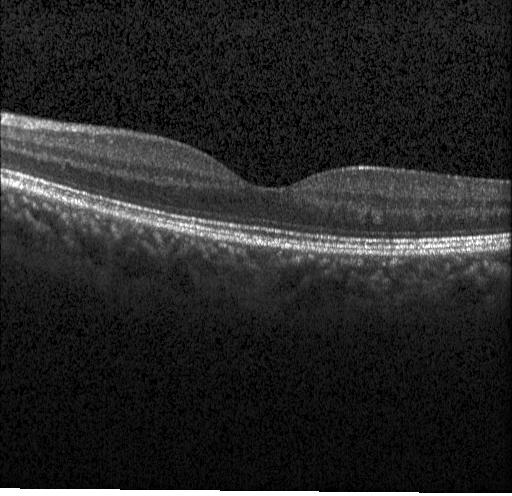 Spectral-domain OCT. Acquired on a Heidelberg Spectralis. Through the macula. Retinal OCT B-scan
This B-scan demonstrates no CNV, no DME, and no drusen.